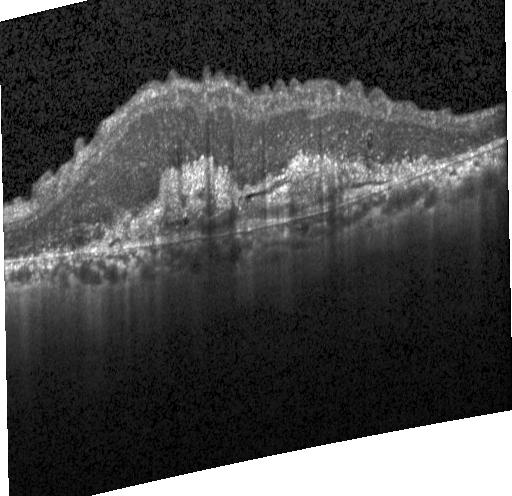 This B-scan demonstrates a choroidal neovascular membrane.